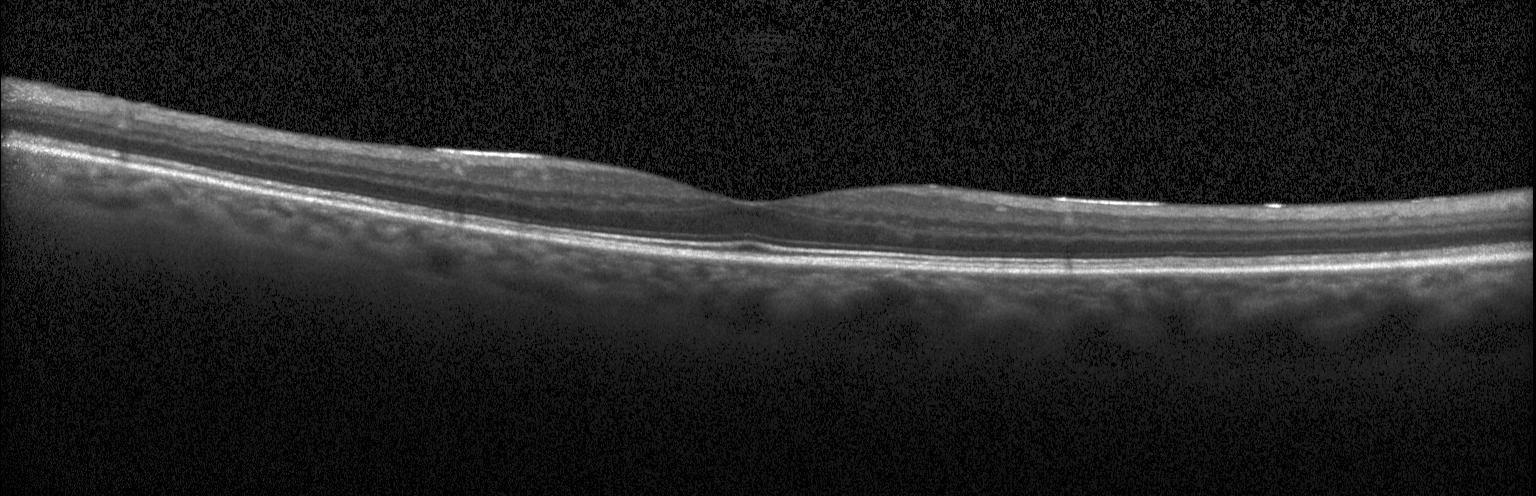 Heidelberg Spectralis. Spectral-domain OCT. Retinal OCT B-scan. Centered on the fovea. Impression: no CNV, no DME, and no drusen.